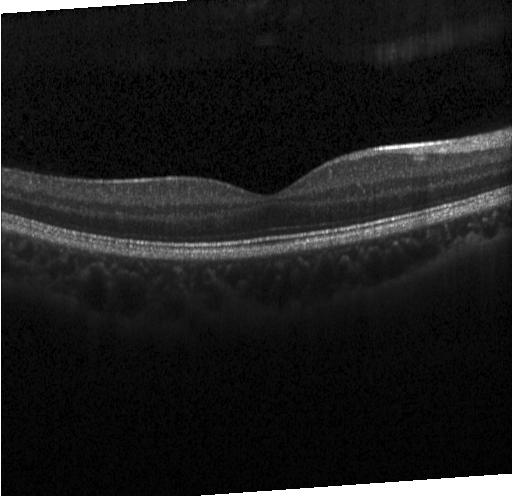

Instrument: Heidelberg Spectralis; retinal OCT B-scan; macular scan; spectral-domain optical coherence tomography
Diagnosis: neither choroidal neovascularization, diabetic macular edema, nor drusen.